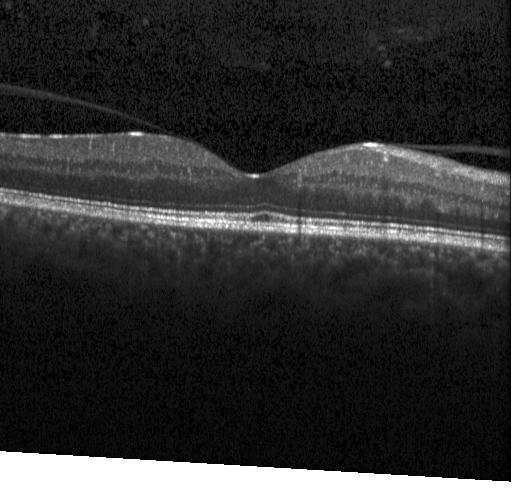
Spectral-domain OCT. Optical coherence tomography B-scan
Assessment: no choroidal neovascularization, diabetic macular edema, or drusen.